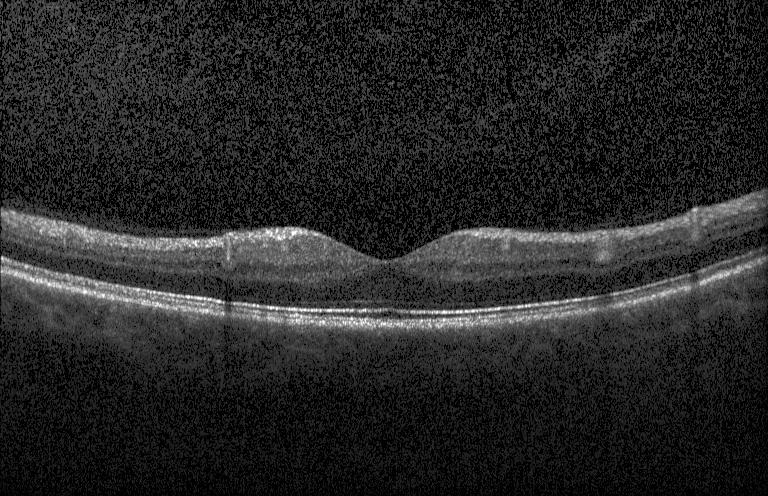 Through the macula. Heidelberg Spectralis. OCT B-scan. Spectral-domain optical coherence tomography
Assessment: no choroidal neovascularization, diabetic macular edema, or drusen.